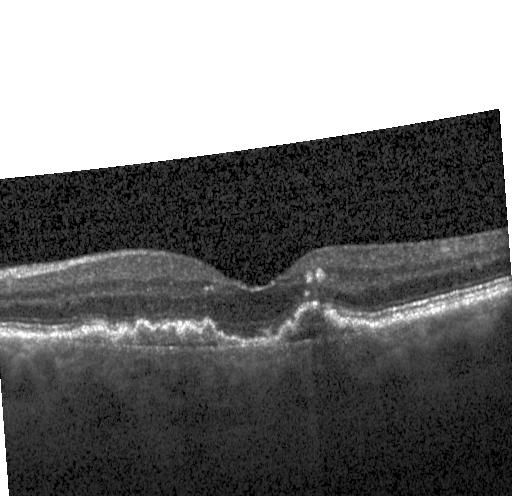
Retinal OCT B-scan
Finding: CNV.